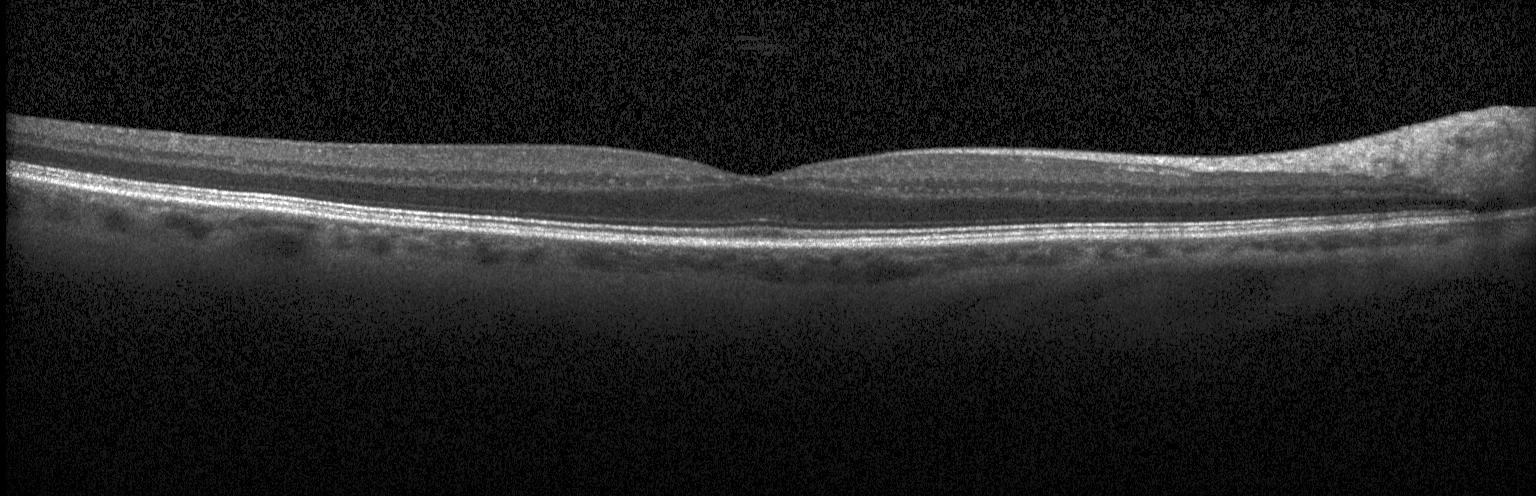

Spectral-domain OCT, fovea-centered, Heidelberg Spectralis OCT system, OCT B-scan. Impression: no choroidal neovascularization, diabetic macular edema, or drusen.